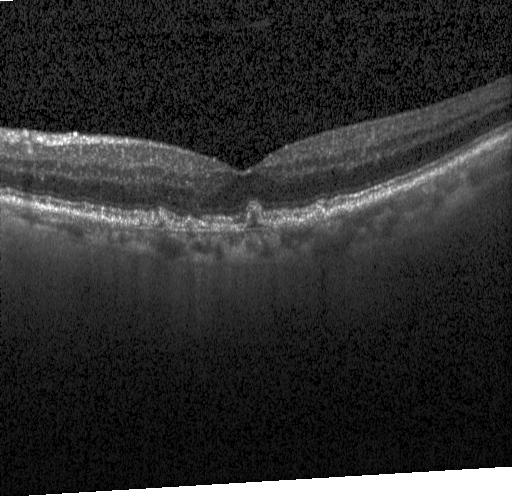

Impression: CNV.